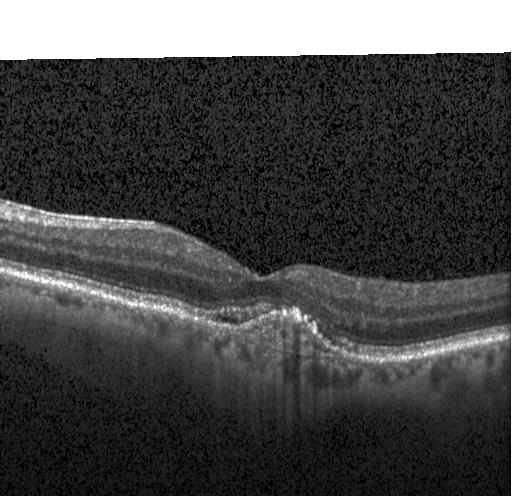

Optical coherence tomography B-scan. Fovea-centered. Heidelberg Spectralis
Diagnosis: CNV.